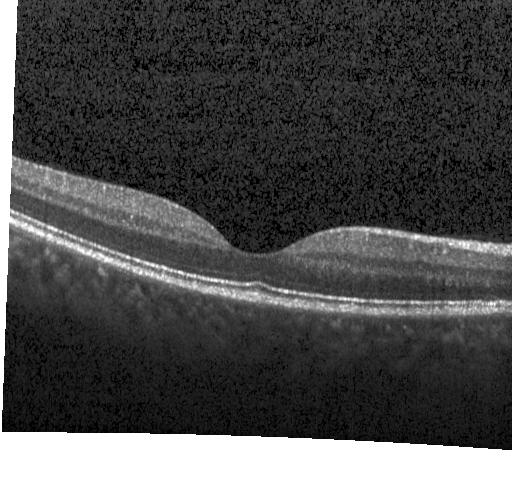
Dx: neither choroidal neovascularization, diabetic macular edema, nor drusen.